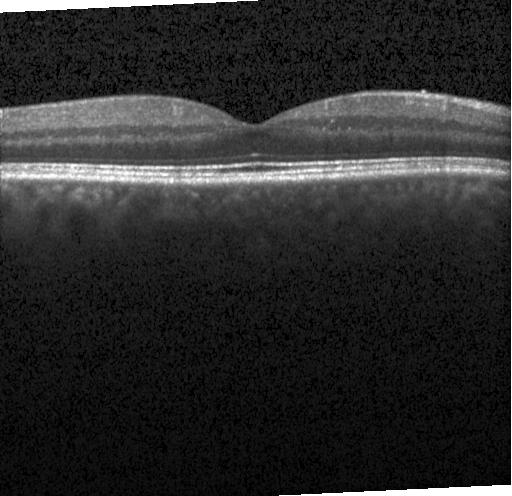 Spectral-domain optical coherence tomography. OCT B-scan. Through the macula.
Diagnosis: no evidence of choroidal neovascularization, diabetic macular edema, or drusen.